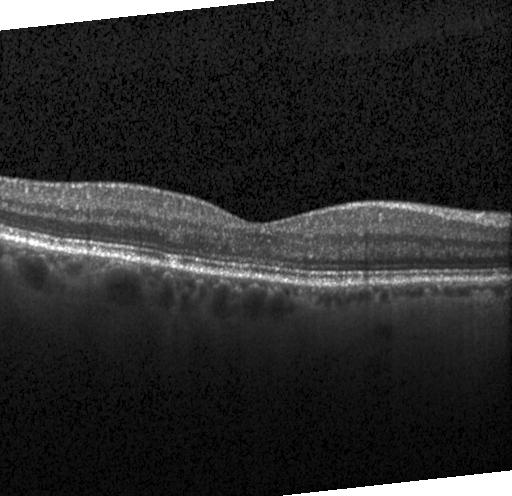 No evidence of CNV, DME, or drusen.